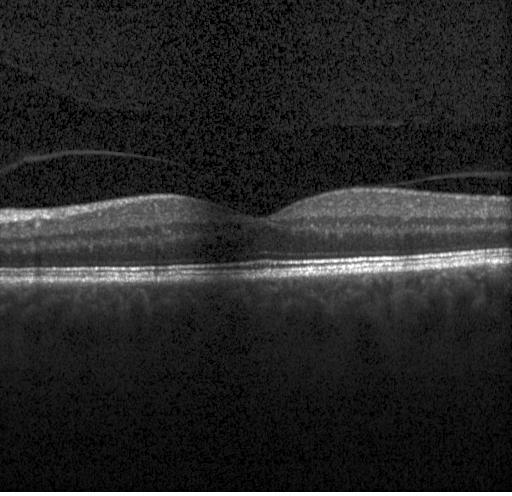
Instrument: Heidelberg Spectralis, SD-OCT, through the macula, optical coherence tomography scan
No CNV, DME, or drusen.